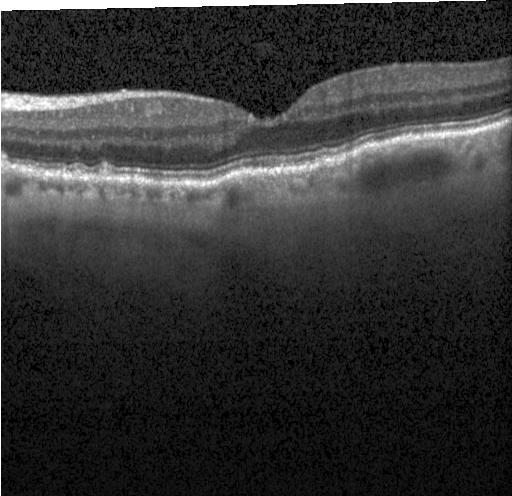 Horizontal scan through the fovea. Spectral-domain OCT. Optical coherence tomography B-scan. OCT finding: multiple drusen.